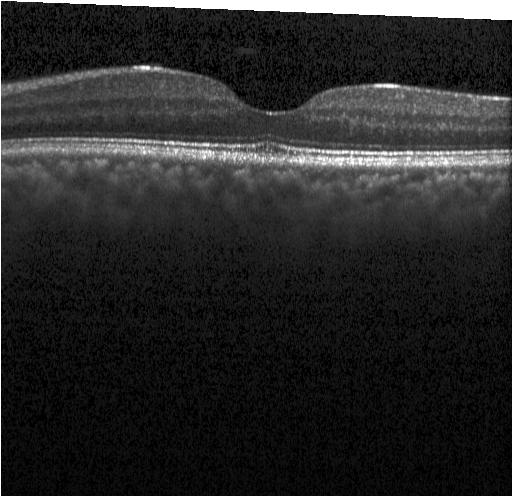

OCT finding: no choroidal neovascularization, no diabetic macular edema, and no drusen.